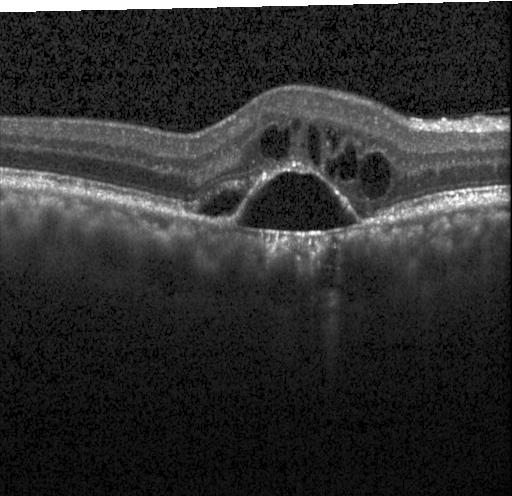

Macular scan · spectral-domain OCT · acquired on a Heidelberg Spectralis · optical coherence tomography B-scan — Diagnosis: CNV.